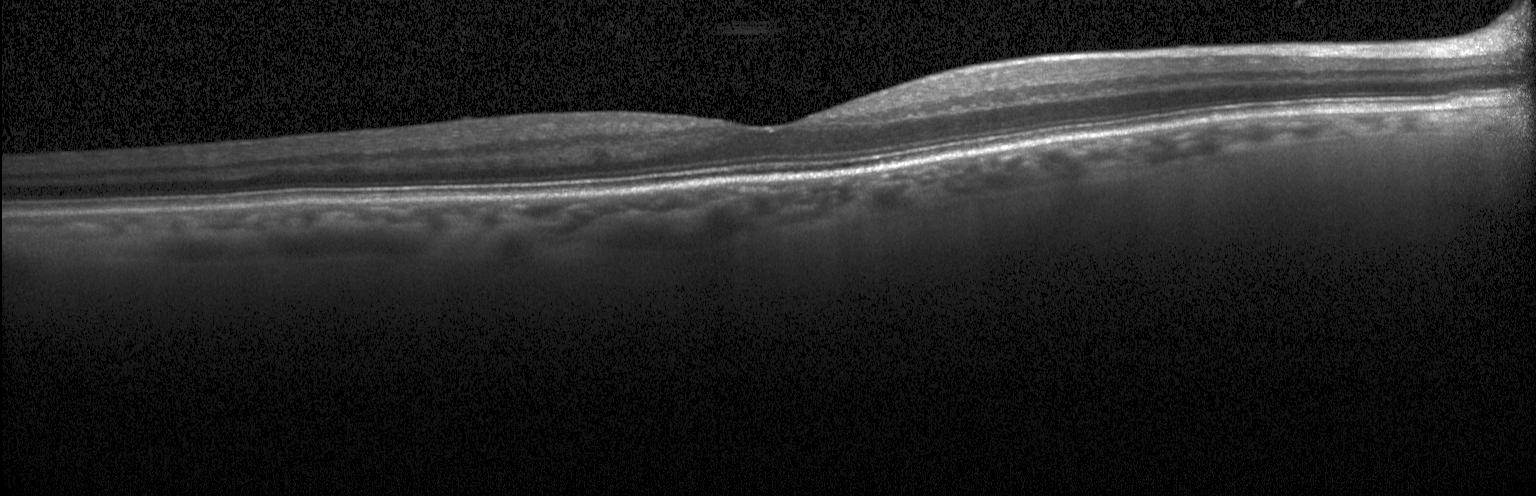 OCT scan showing no CNV, no DME, and no drusen.